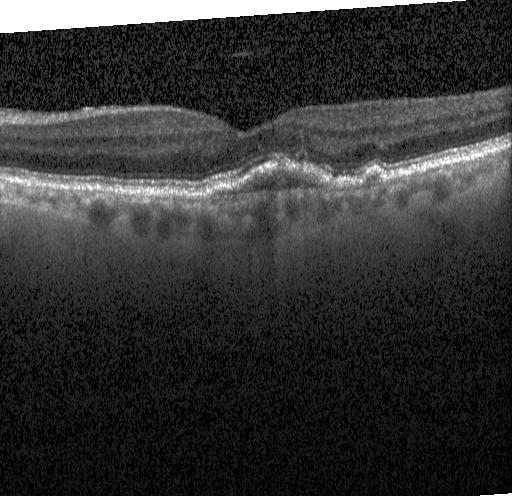

Through the macula; acquired on a Heidelberg Spectralis; OCT B-scan
The scan shows choroidal neovascularization.